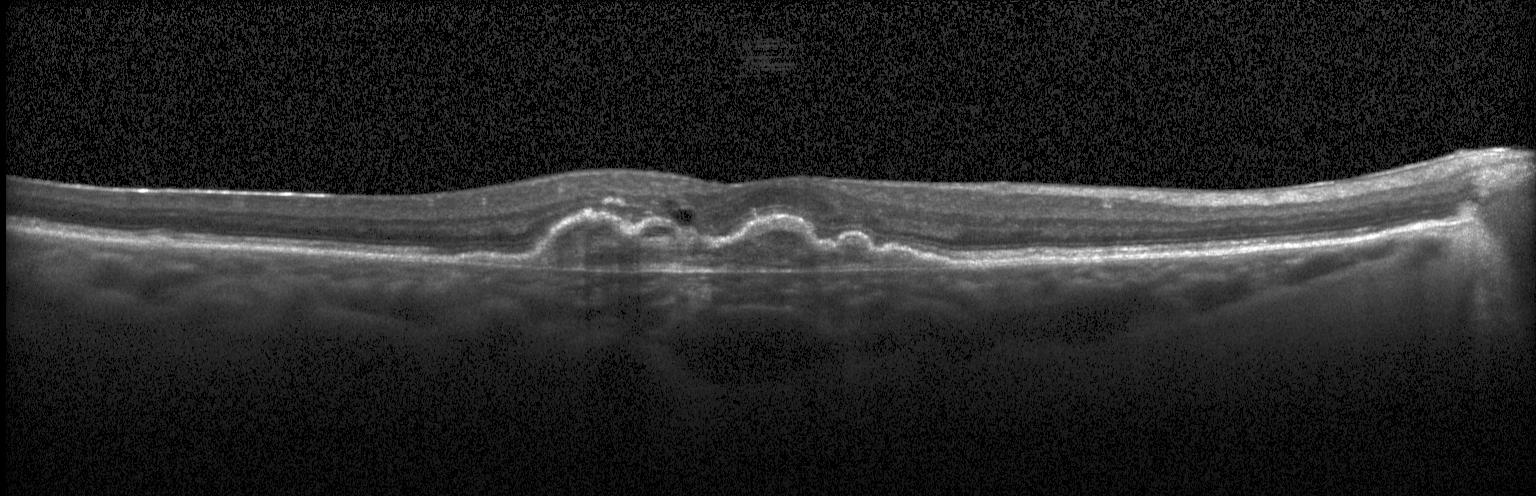
Fovea-centered · optical coherence tomography scan
Finding: a choroidal neovascular membrane.